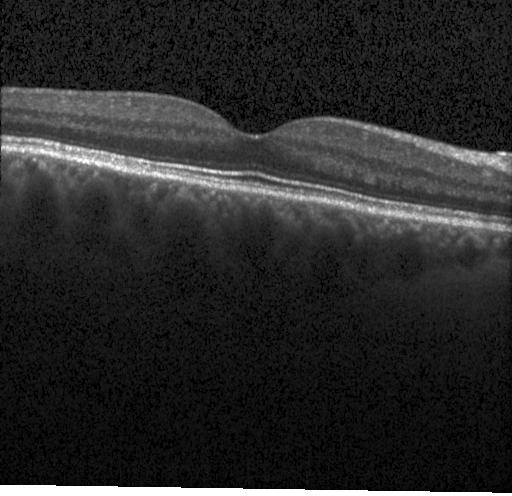
Diagnosis: no evidence of choroidal neovascularization, diabetic macular edema, or drusen.